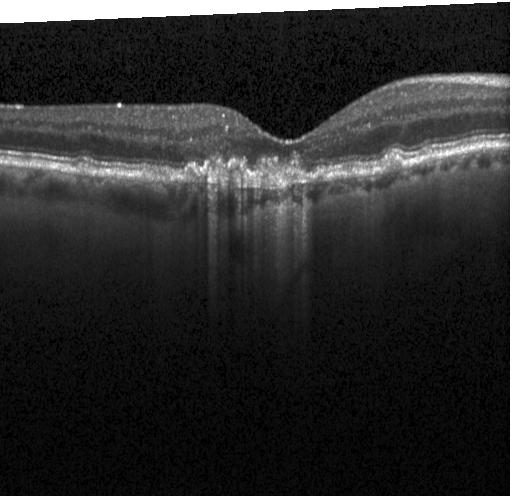

Instrument: Heidelberg Spectralis. Retinal OCT cross-section — Diagnosis: a choroidal neovascular membrane.